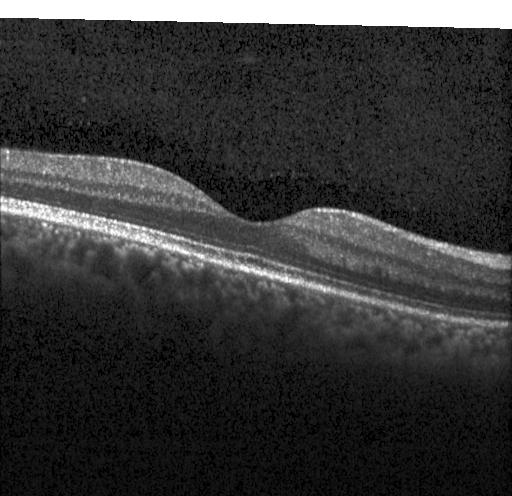

Finding: neither CNV, DME, nor drusen.